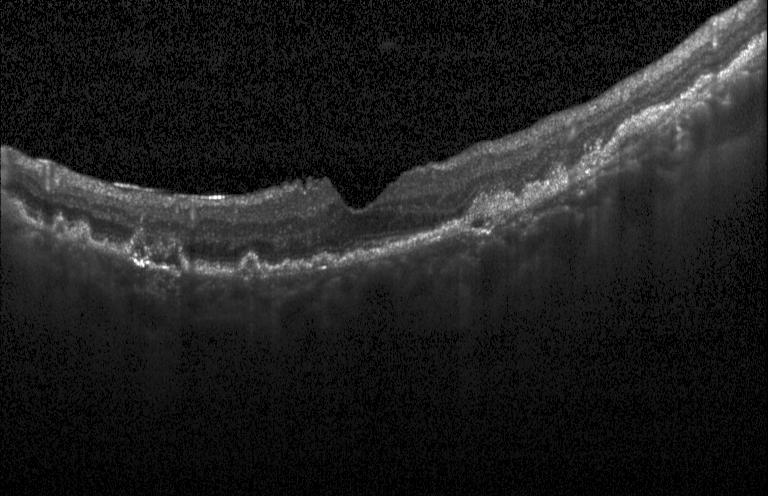
OCT B-scan showing a choroidal neovascular membrane.